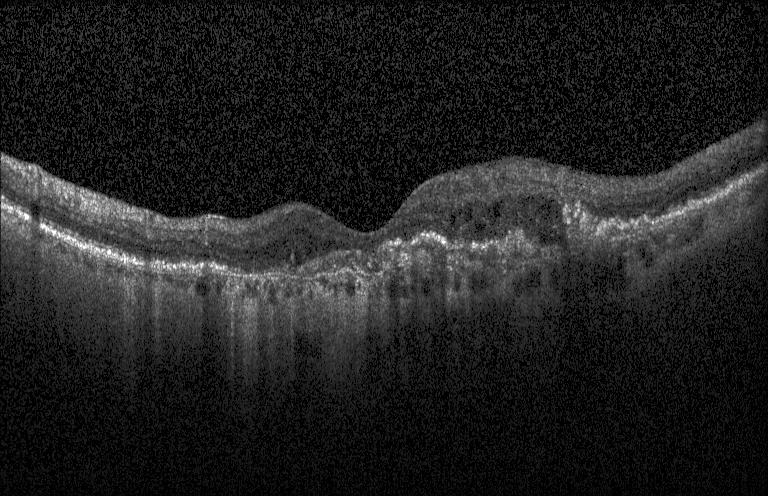 The scan shows choroidal neovascularization (CNV).